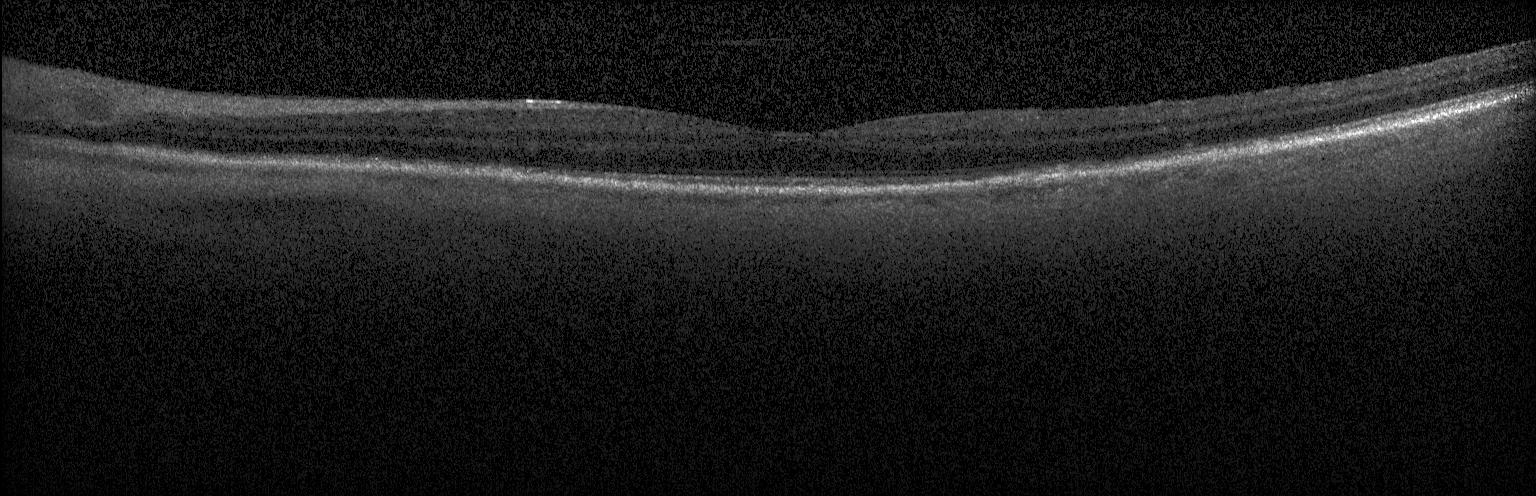

SD-OCT, optical coherence tomography scan
Diagnosis: neither choroidal neovascularization, diabetic macular edema, nor drusen.